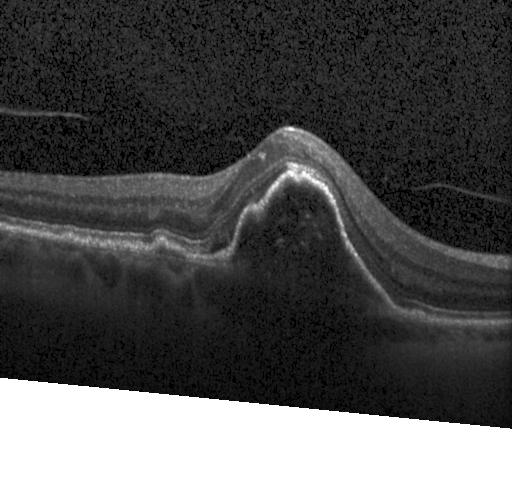 The scan shows a choroidal neovascular membrane.